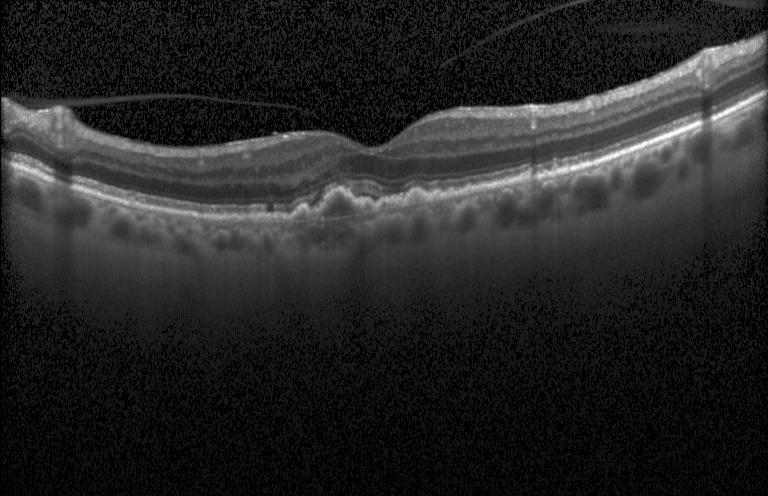 Assessment: a choroidal neovascular membrane.